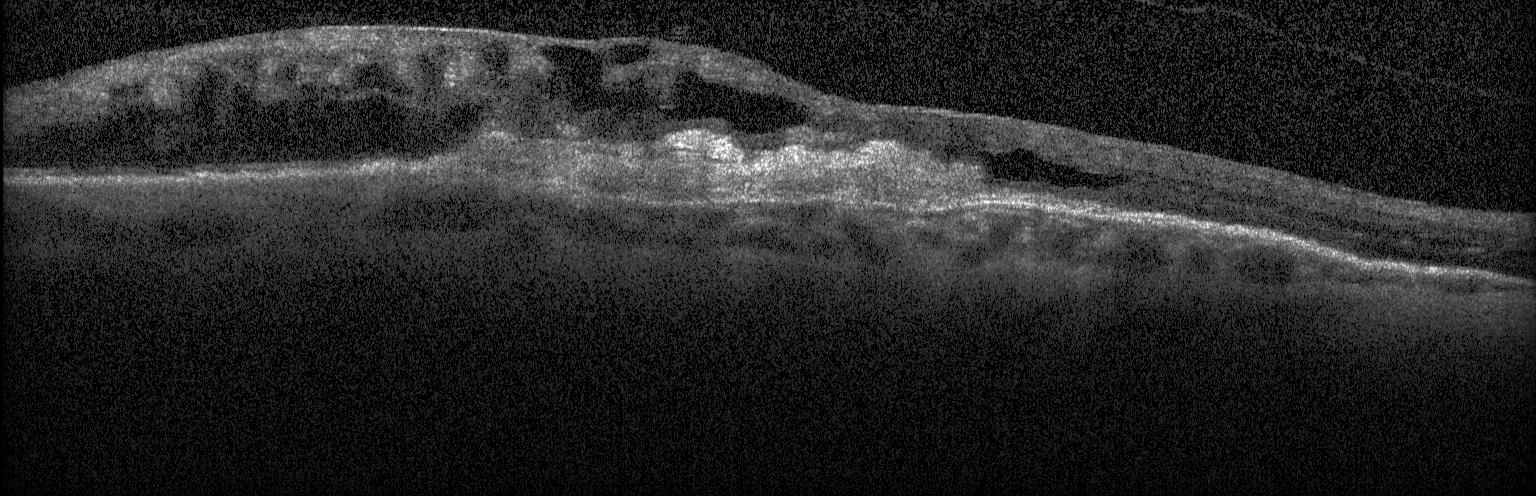 SD-OCT; OCT B-scan — Assessment: choroidal neovascularization.